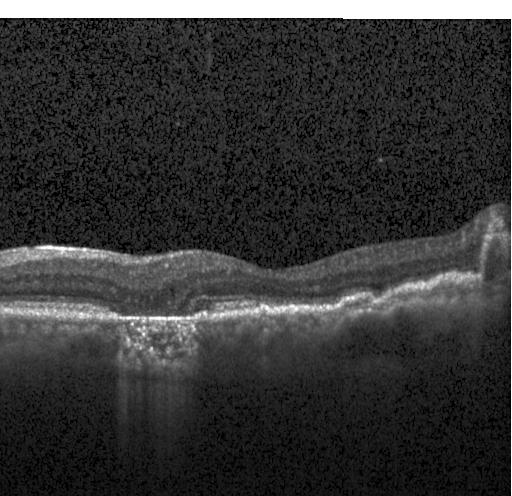 Dx: choroidal neovascularization.